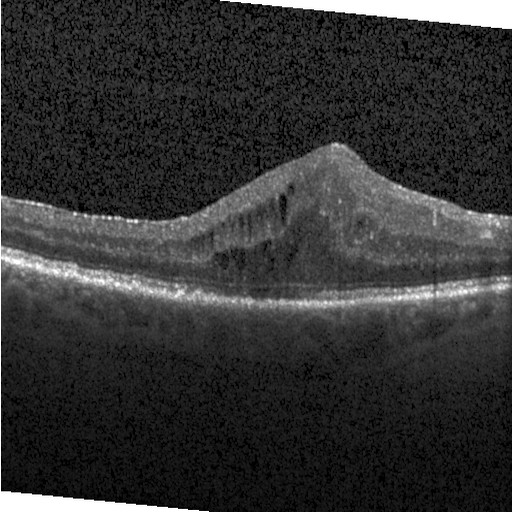 Spectral-domain optical coherence tomography; Heidelberg Spectralis OCT system; retinal OCT cross-section.
This B-scan demonstrates diabetic macular edema (DME).